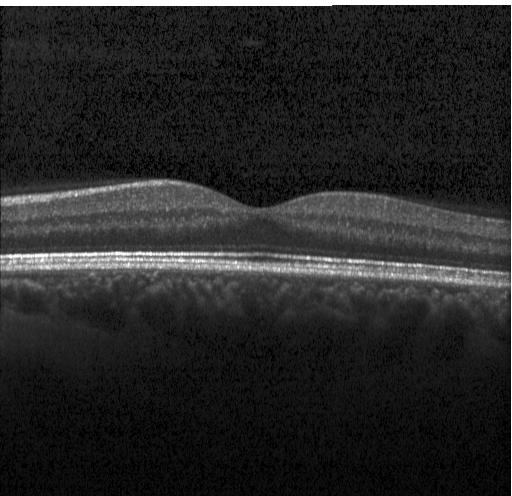

OCT B-scan showing no evidence of choroidal neovascularization, diabetic macular edema, or drusen.